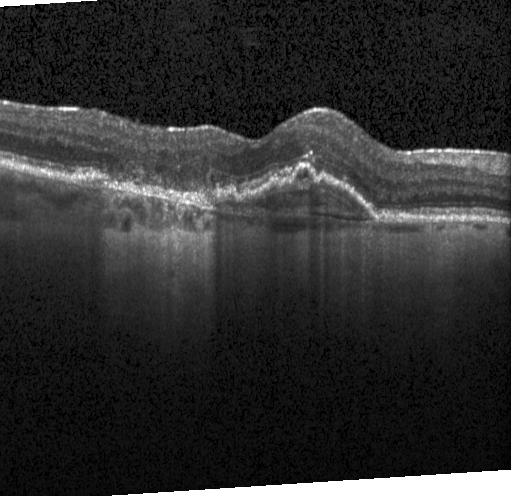
OCT B-scan; acquired on a Heidelberg Spectralis; spectral-domain optical coherence tomography. Diagnosis: choroidal neovascularization.